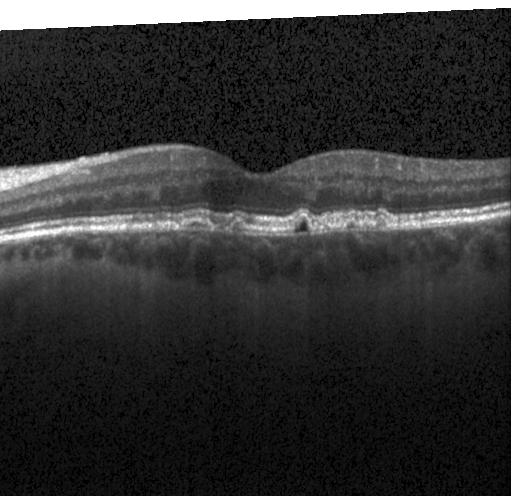 Spectral-domain OCT; acquired on a Heidelberg Spectralis; optical coherence tomography scan.
Assessment: drusen.